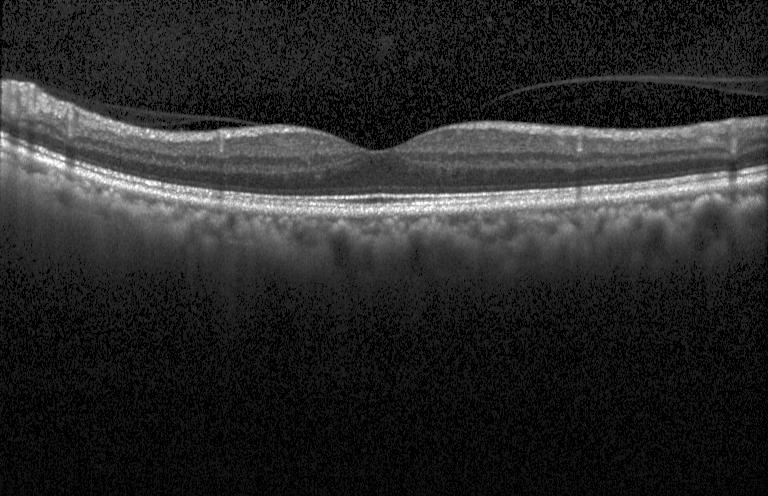 Dx: no CNV, no DME, and no drusen.